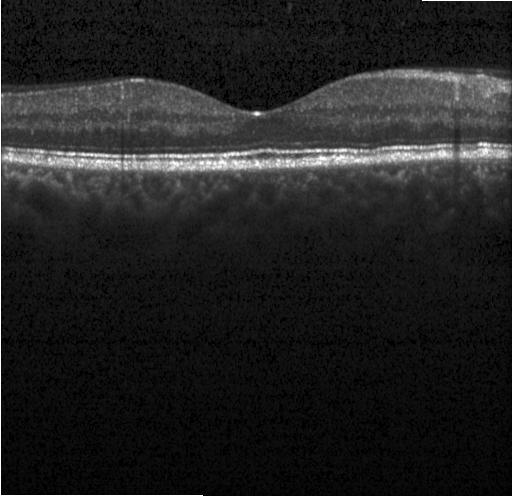
OCT line scan · centered on the fovea · Heidelberg Spectralis
Diagnosis: no choroidal neovascularization, no diabetic macular edema, and no drusen.